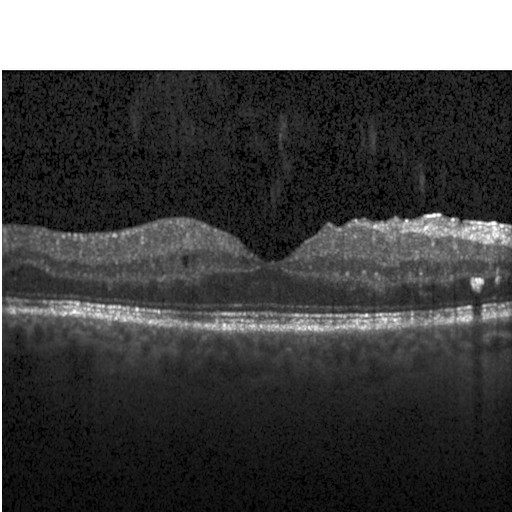 The scan shows diabetic macular edema.